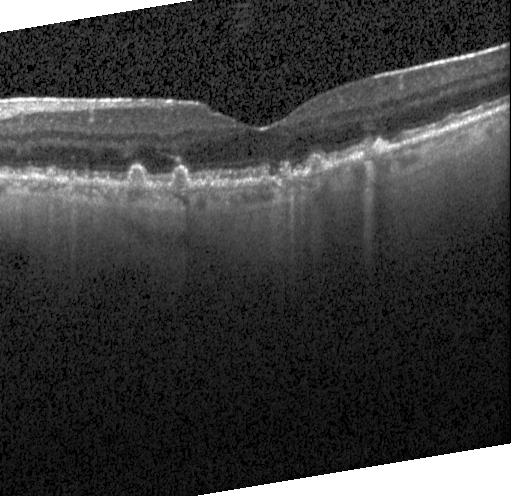

Spectral-domain OCT B-scan: drusen.